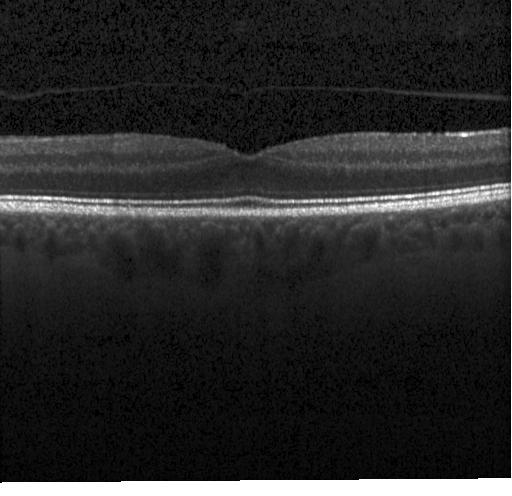

Through the macula · optical coherence tomography B-scan. Finding: no evidence of CNV, DME, or drusen.